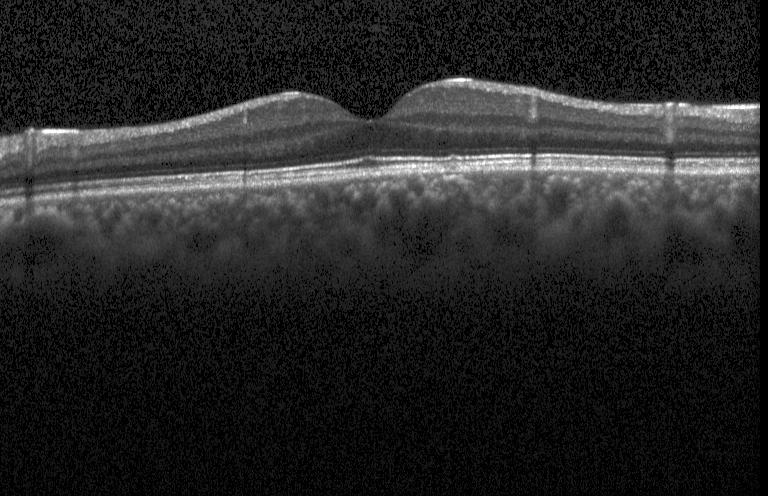 Finding: no evidence of choroidal neovascularization, diabetic macular edema, or drusen.